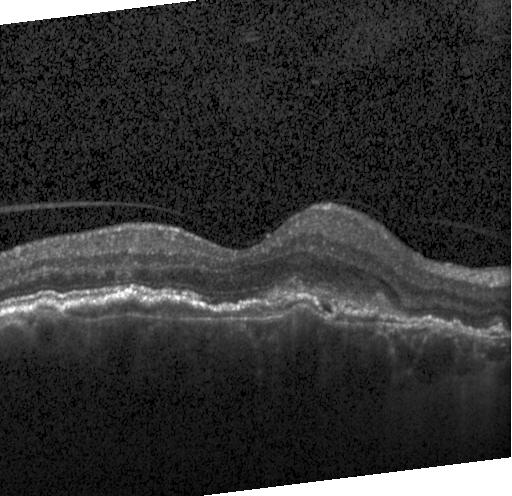 The scan shows a choroidal neovascular membrane.